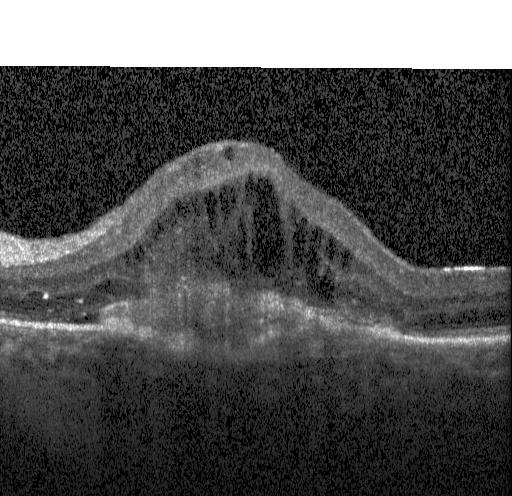
Diagnosis: choroidal neovascularization (CNV).